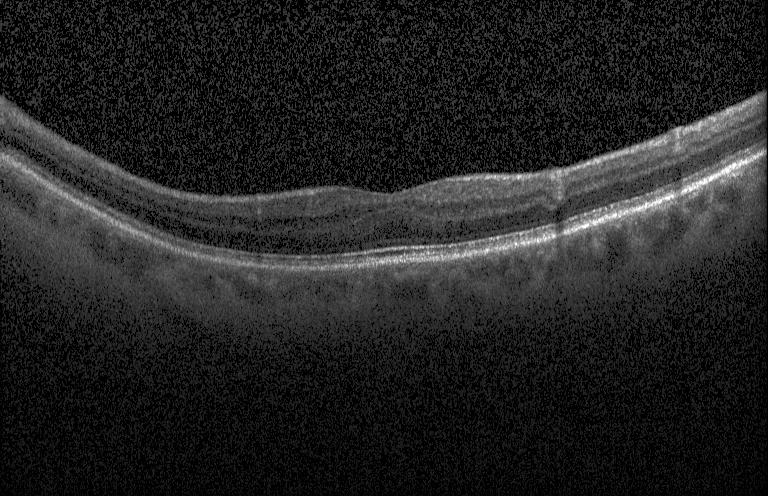
Heidelberg Spectralis OCT system; OCT B-scan
No evidence of CNV, DME, or drusen.